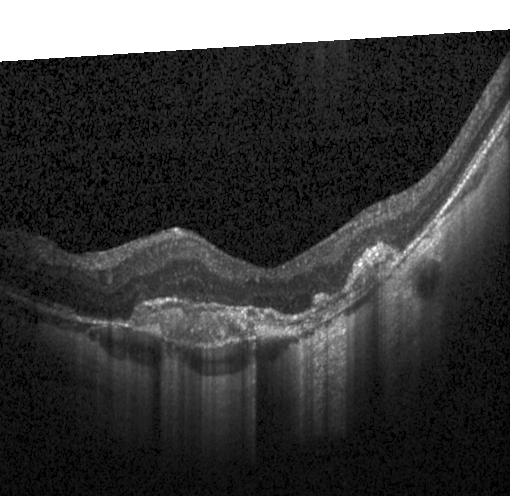 Centered on the fovea; spectral-domain optical coherence tomography; optical coherence tomography B-scan. Assessment: a choroidal neovascular membrane.